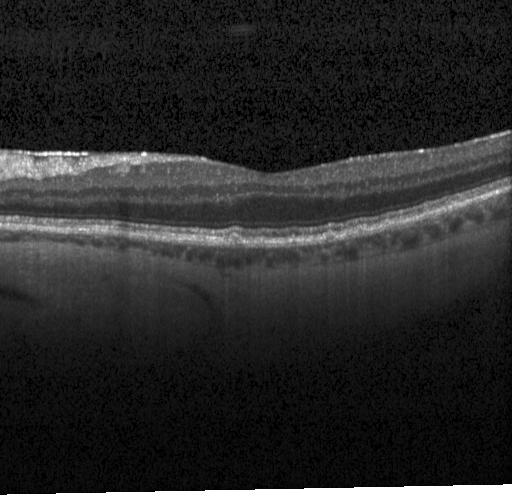

Macular OCT demonstrating sub-RPE drusenoid deposits.